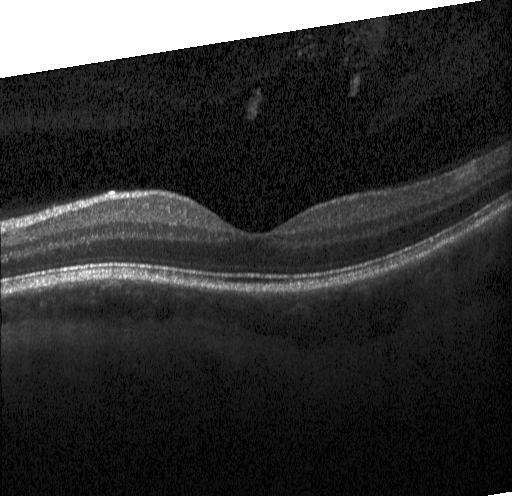
Retinal OCT cross-section — Macular OCT: no evidence of choroidal neovascularization, diabetic macular edema, or drusen.